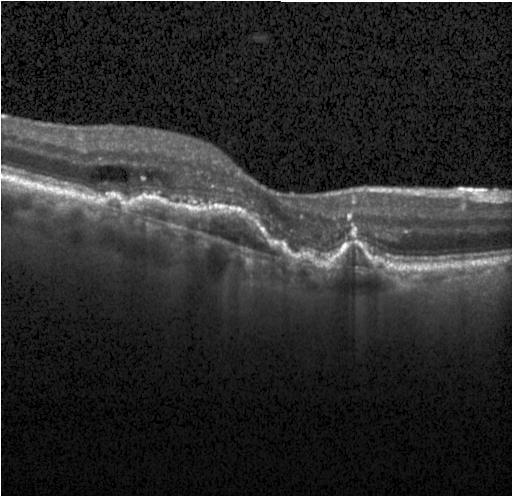 OCT finding: a choroidal neovascular membrane.